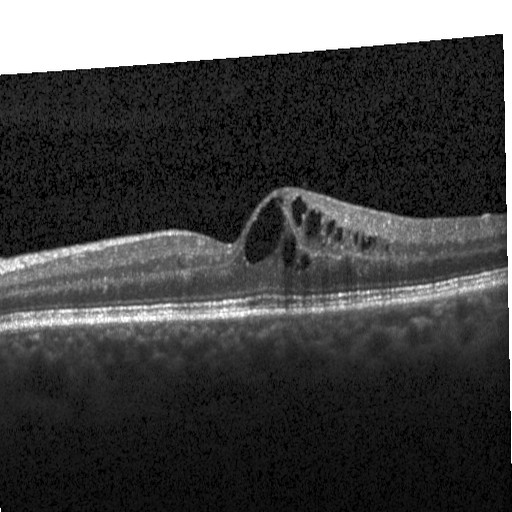 Spectral-domain OCT; retinal OCT B-scan — Finding: diabetic macular edema.